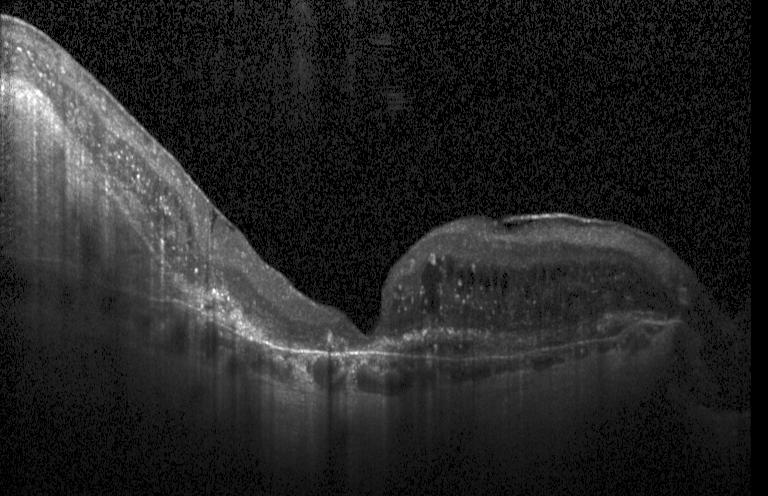
Dx: a choroidal neovascular membrane.